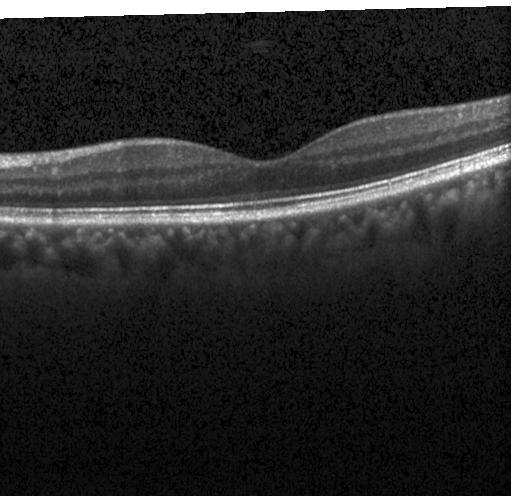

Optical coherence tomography B-scan; Heidelberg Spectralis; SD-OCT; through the macula.
This B-scan demonstrates no evidence of choroidal neovascularization, diabetic macular edema, or drusen.